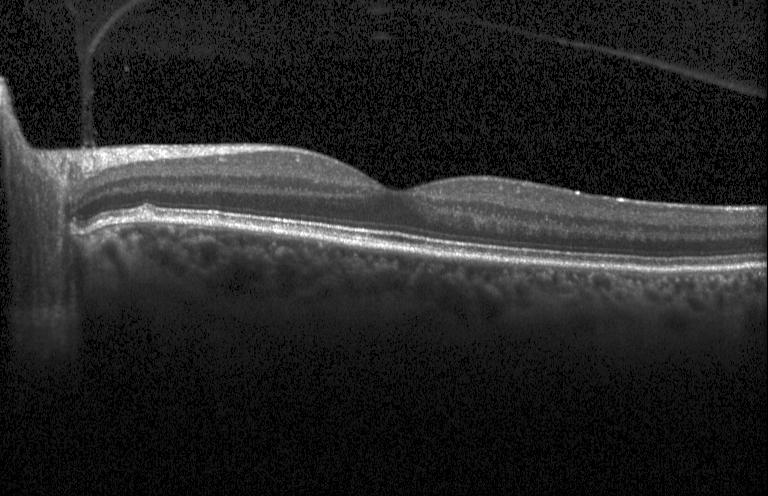 Retinal OCT cross-section showing drusen.